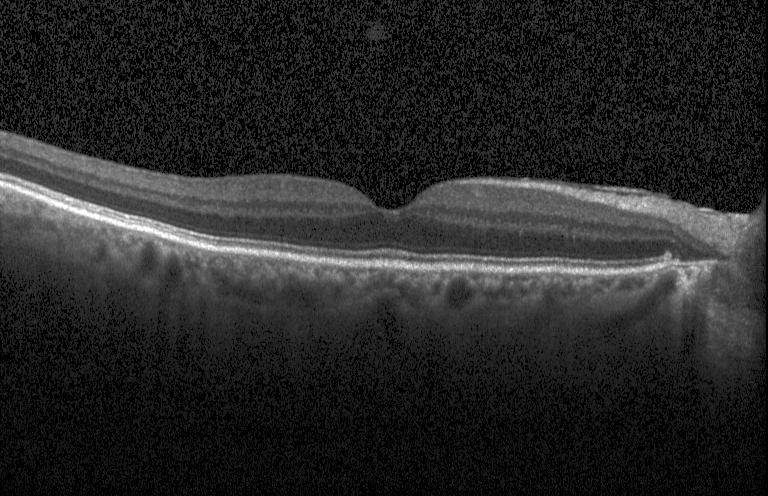
Optical coherence tomography B-scan; acquired on a Heidelberg Spectralis; horizontal scan through the fovea; spectral-domain OCT. This B-scan demonstrates no evidence of CNV, DME, or drusen.